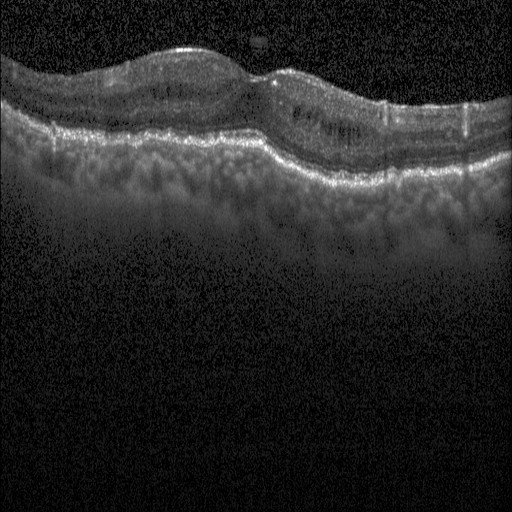
Optical coherence tomography B-scan — This B-scan demonstrates diabetic macular edema.